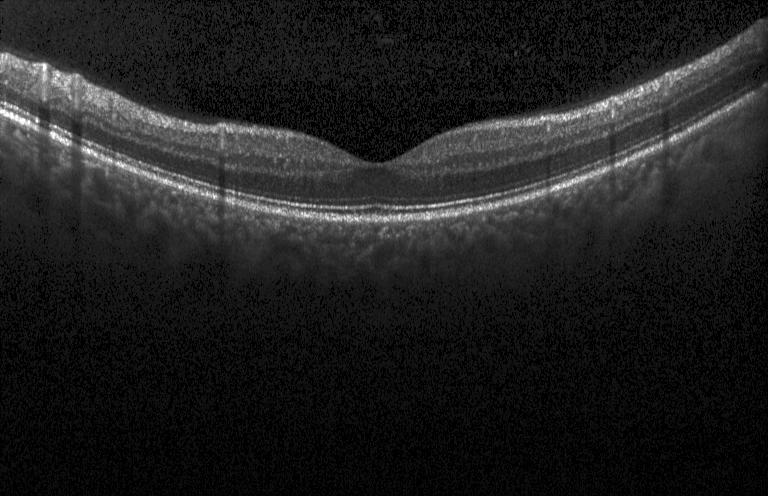 OCT B-scan. Heidelberg Spectralis. SD-OCT — Finding: no evidence of choroidal neovascularization, diabetic macular edema, or drusen.